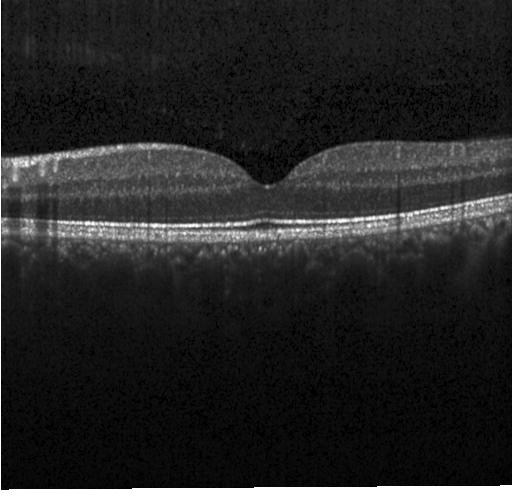 OCT line scan, spectral-domain OCT, fovea-centered. Impression: neither choroidal neovascularization, diabetic macular edema, nor drusen.